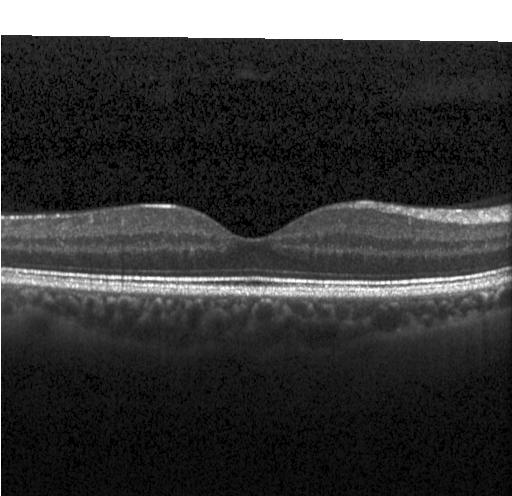
Spectral-domain OCT; retinal OCT cross-section; instrument: Heidelberg Spectralis; through the macula — This B-scan demonstrates no evidence of choroidal neovascularization, diabetic macular edema, or drusen.